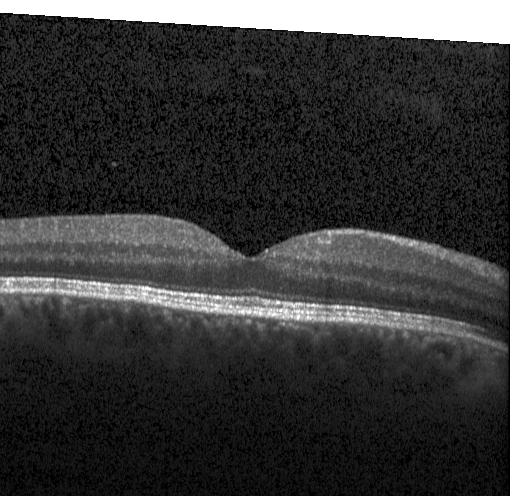
Retinal OCT B-scan. This B-scan demonstrates no CNV, DME, or drusen.